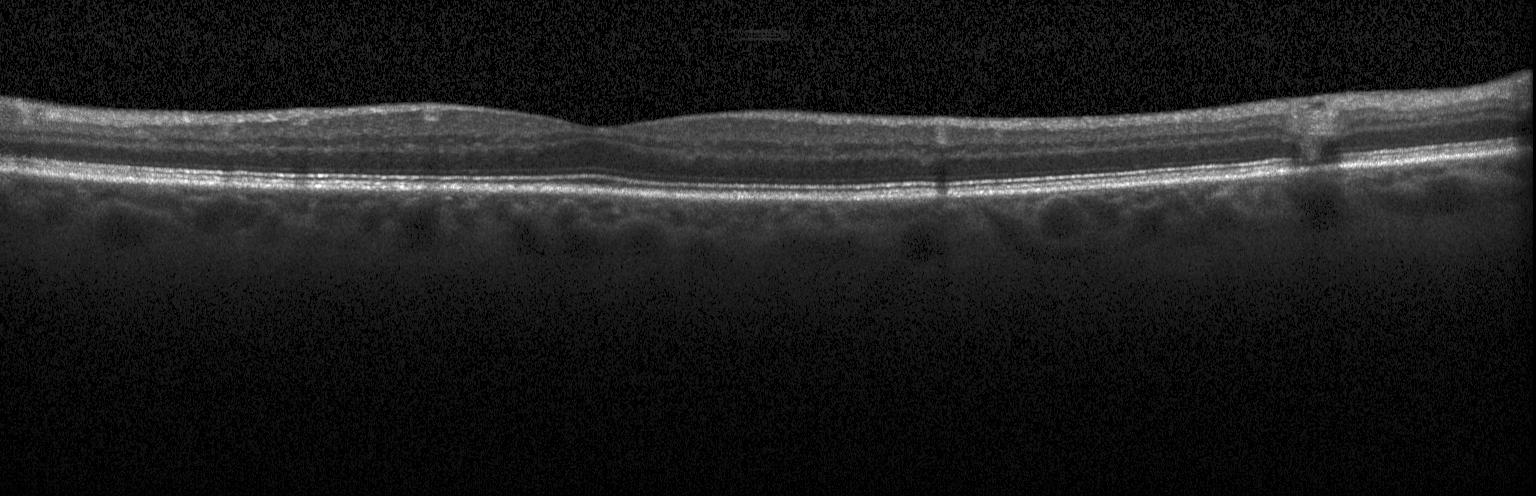 OCT line scan. Fovea-centered. Acquired on a Heidelberg Spectralis.
Impression: no choroidal neovascularization, diabetic macular edema, or drusen.